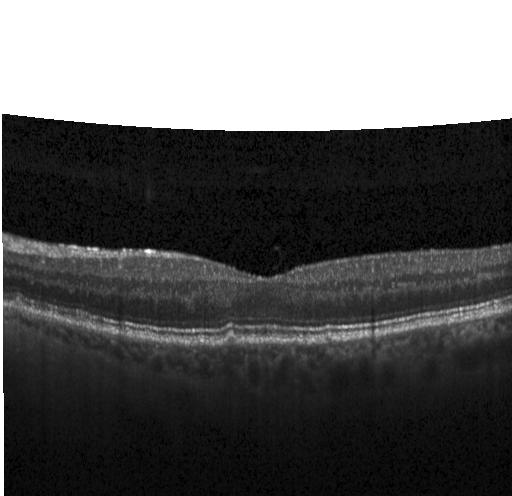 SD-OCT, centered on the fovea, retinal OCT cross-section. OCT finding: sub-RPE drusenoid deposits.